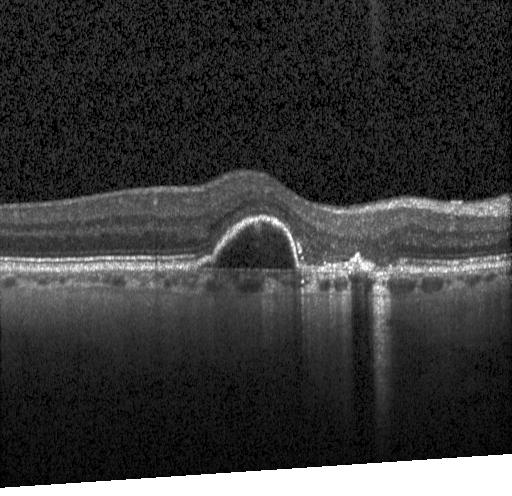
Horizontal scan through the fovea. Spectral-domain OCT. Retinal OCT cross-section. Instrument: Heidelberg Spectralis — Finding: a choroidal neovascular membrane.